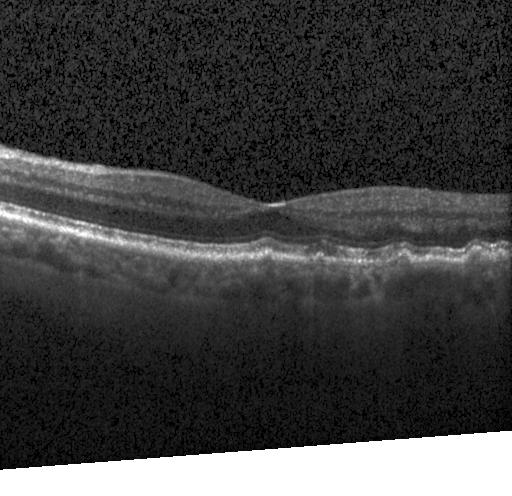

Finding: sub-RPE drusenoid deposits.